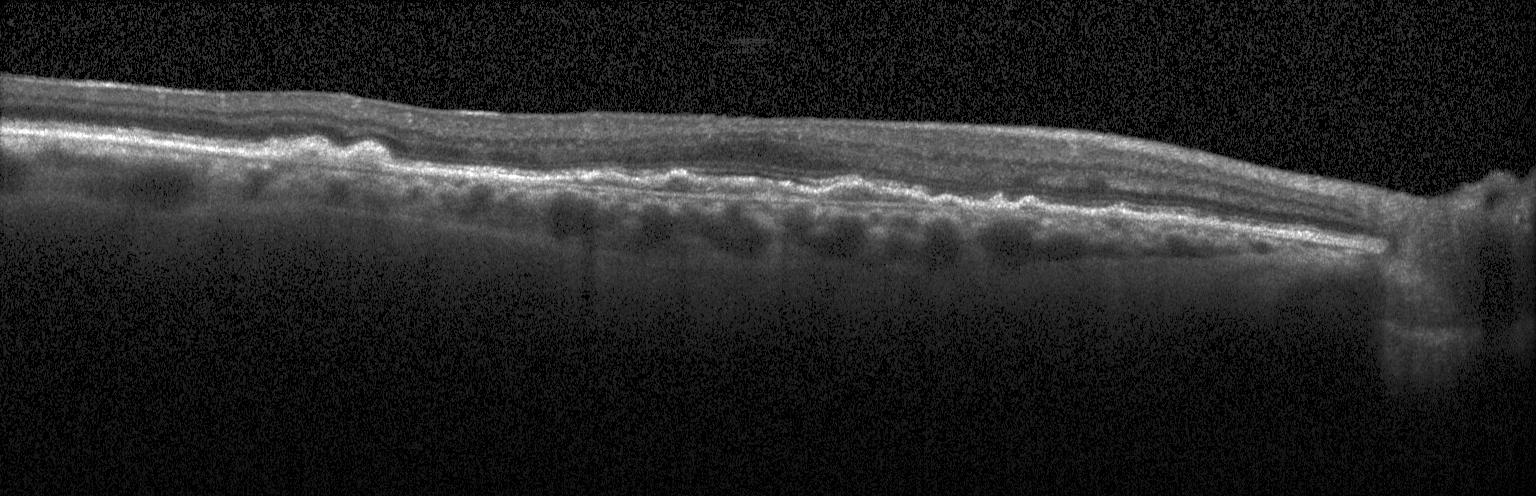

Macular scan, SD-OCT, retinal OCT cross-section — A choroidal neovascular membrane.